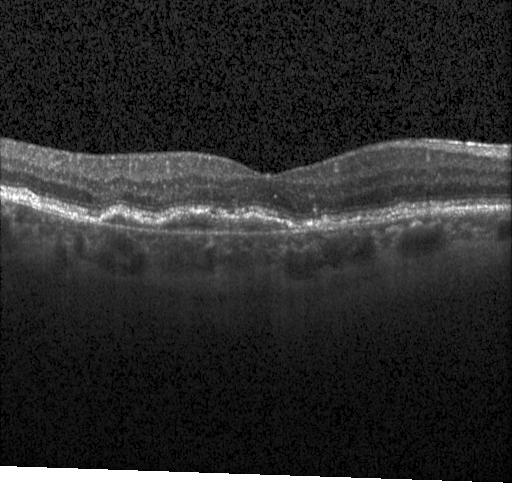 Finding: a choroidal neovascular membrane.